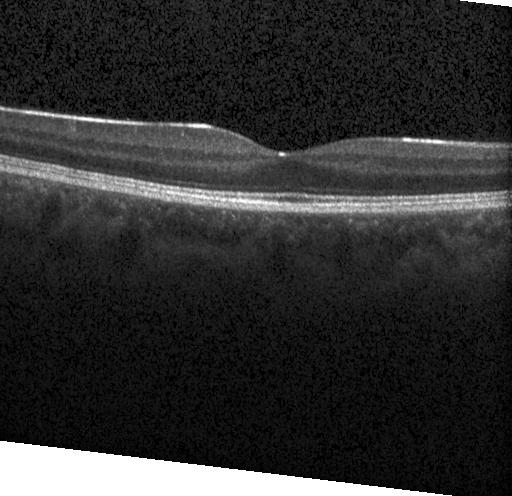 Fovea-centered · spectral-domain optical coherence tomography · optical coherence tomography B-scan. Impression: no evidence of CNV, DME, or drusen.